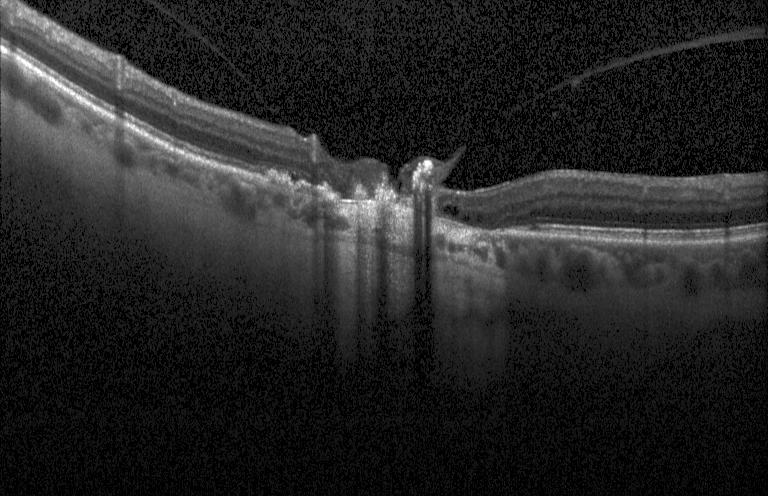

Heidelberg Spectralis; retinal OCT B-scan; spectral-domain OCT. Impression: a choroidal neovascular membrane.